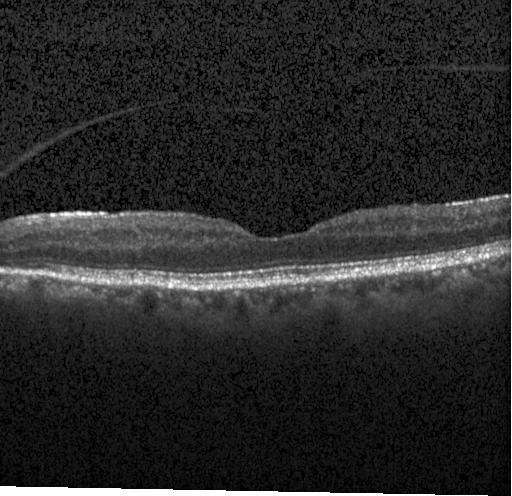

Retinal OCT B-scan — The scan shows neither choroidal neovascularization, diabetic macular edema, nor drusen.